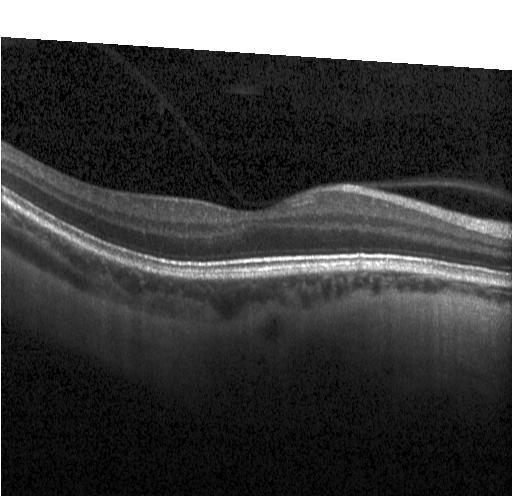
Diagnosis: no evidence of choroidal neovascularization, diabetic macular edema, or drusen.